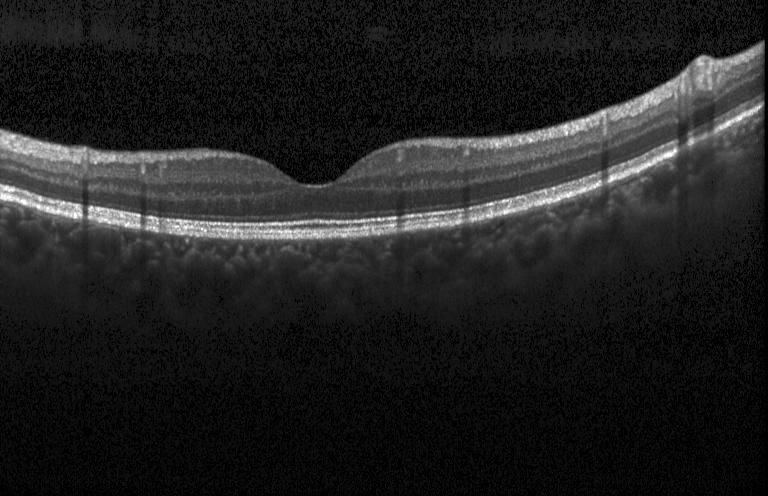 Finding: no CNV, no DME, and no drusen.